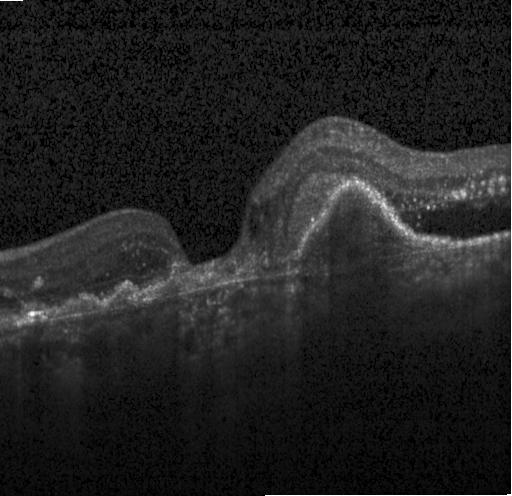 Horizontal scan through the fovea, Heidelberg Spectralis OCT system, optical coherence tomography B-scan — Impression: a choroidal neovascular membrane.